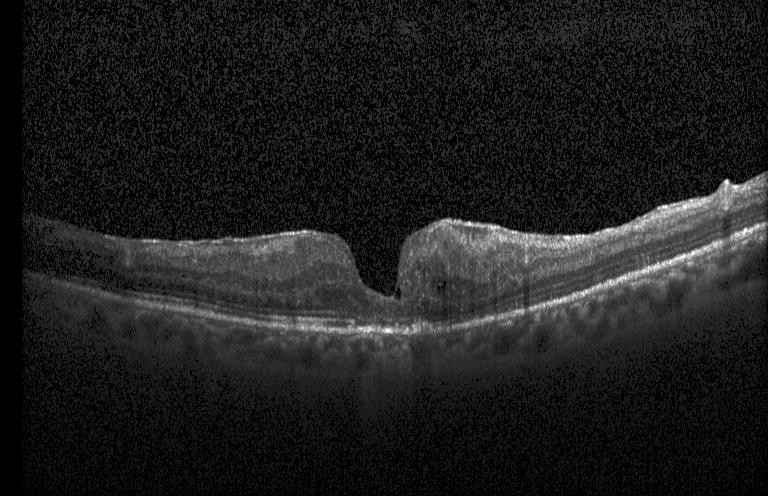 Fovea-centered · retinal OCT B-scan · Heidelberg Spectralis. Assessment: diabetic macular edema (DME).